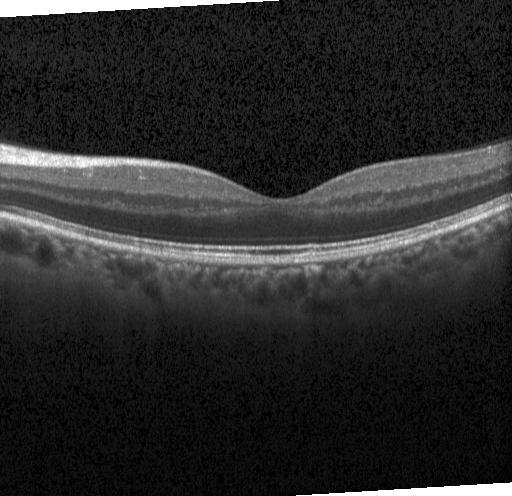

OCT line scan. No choroidal neovascularization, no diabetic macular edema, and no drusen.